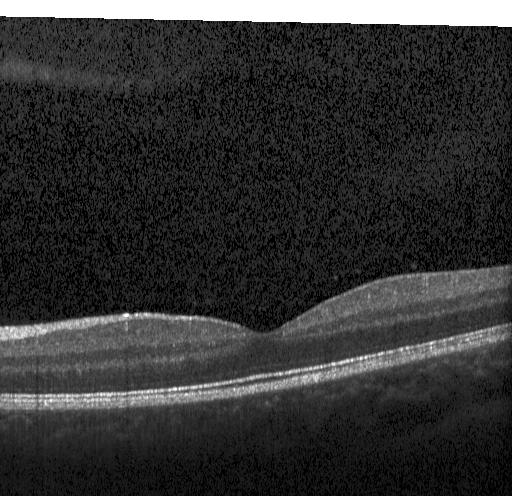
Fovea-centered, spectral-domain optical coherence tomography, Heidelberg Spectralis, retinal OCT B-scan.
This B-scan demonstrates no CNV, no DME, and no drusen.